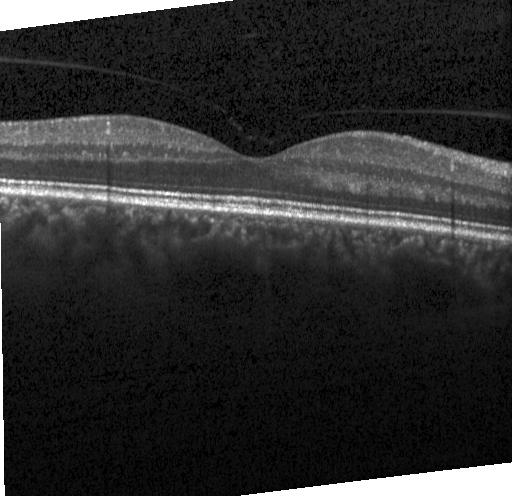
Heidelberg Spectralis, optical coherence tomography B-scan, through the macula, SD-OCT.
Diagnosis: neither CNV, DME, nor drusen.